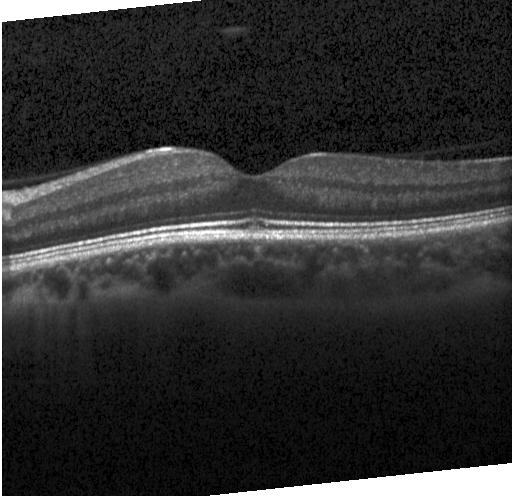
Finding: neither CNV, DME, nor drusen.